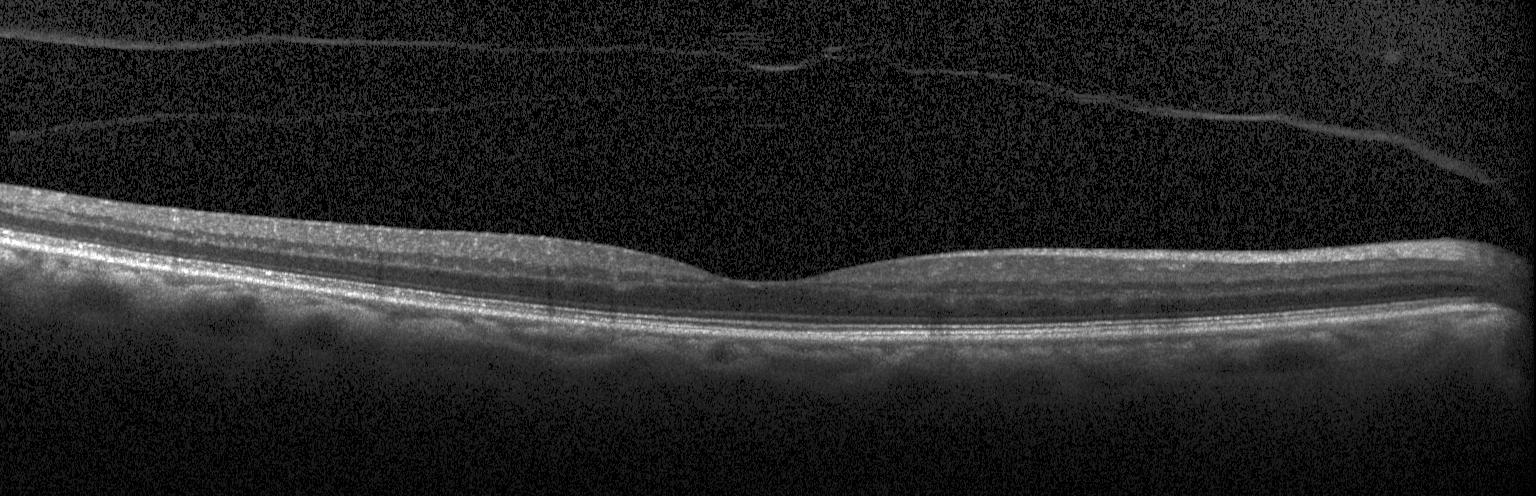 Diagnosis: no CNV, no DME, and no drusen.